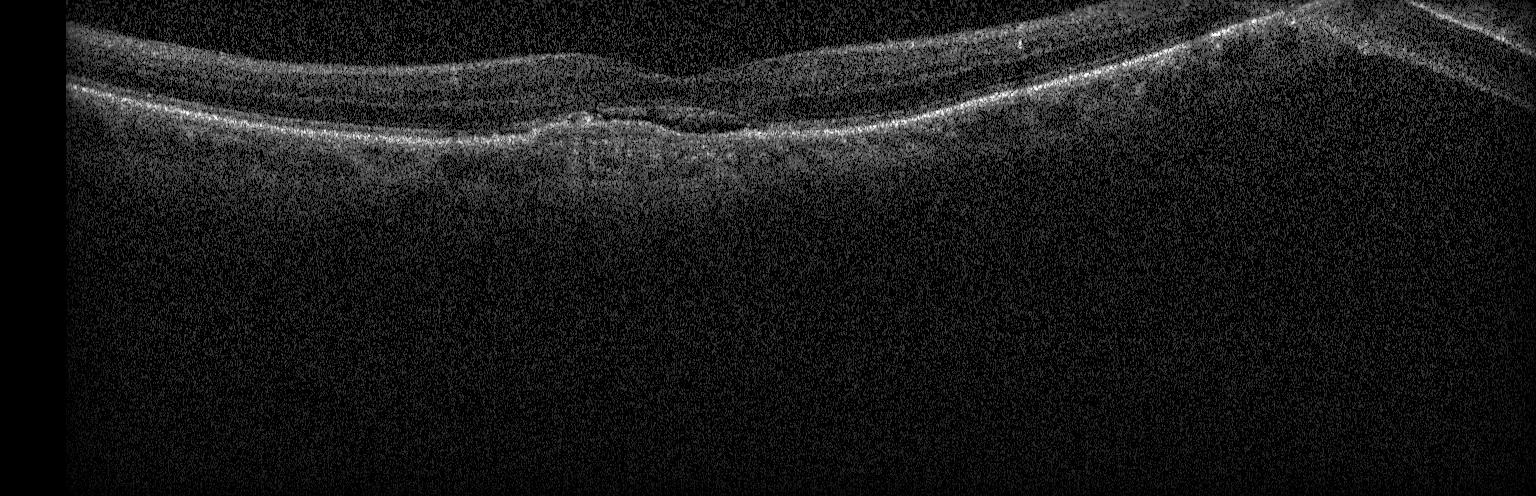
Spectral-domain OCT; optical coherence tomography scan; Heidelberg Spectralis OCT system
Finding: CNV.